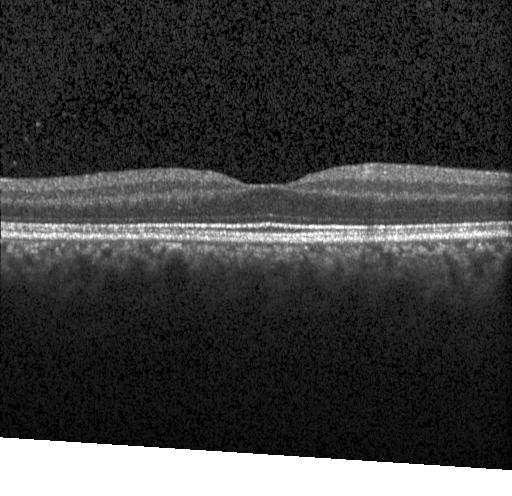
OCT B-scan
Dx: no choroidal neovascularization, diabetic macular edema, or drusen.